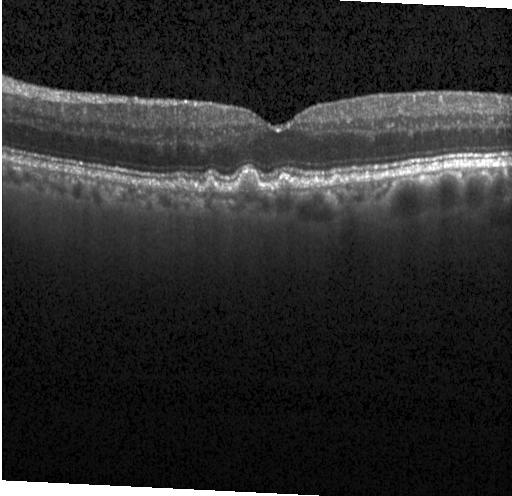

Retinal OCT B-scan · fovea-centered — Macular OCT: drusen.